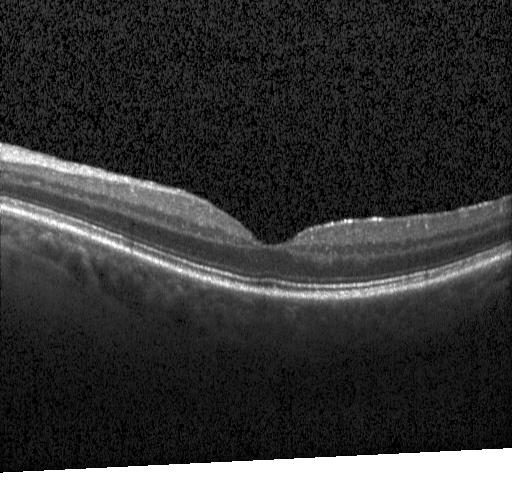
Diagnosis: no choroidal neovascularization, diabetic macular edema, or drusen.